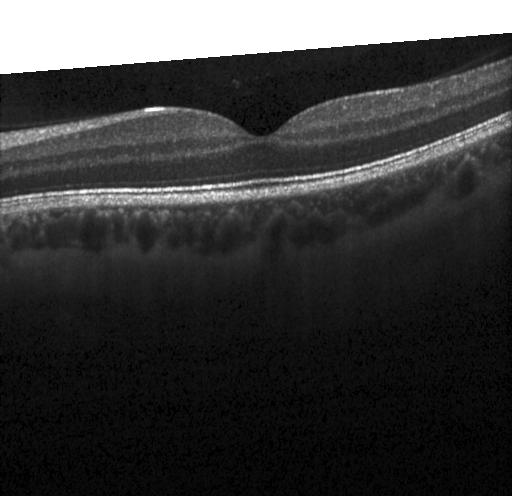 OCT B-scan showing no CNV, no DME, and no drusen.